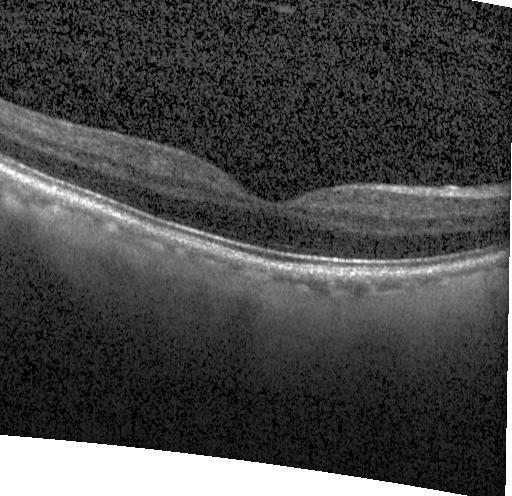

Macular OCT demonstrating no choroidal neovascularization, diabetic macular edema, or drusen.